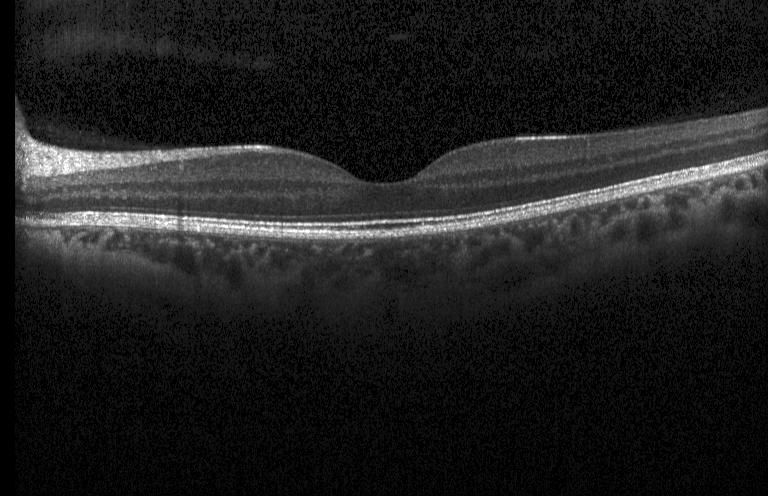

OCT B-scan, fovea-centered. The scan shows no evidence of choroidal neovascularization, diabetic macular edema, or drusen.